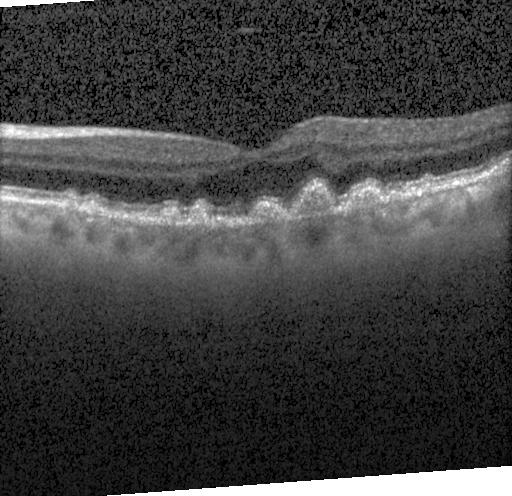
SD-OCT · centered on the fovea · OCT B-scan · instrument: Heidelberg Spectralis
Finding: drusen.